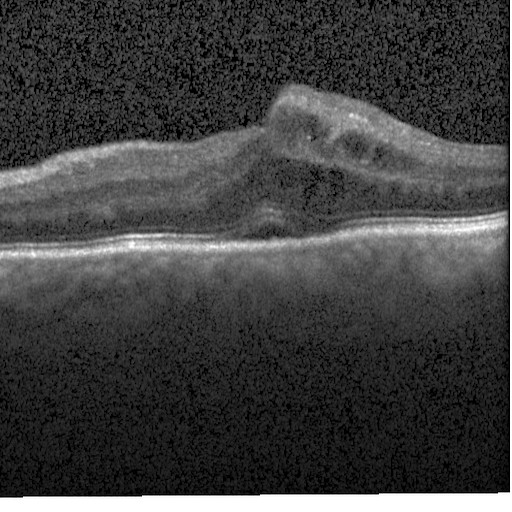

OCT line scan. Dx: DME.